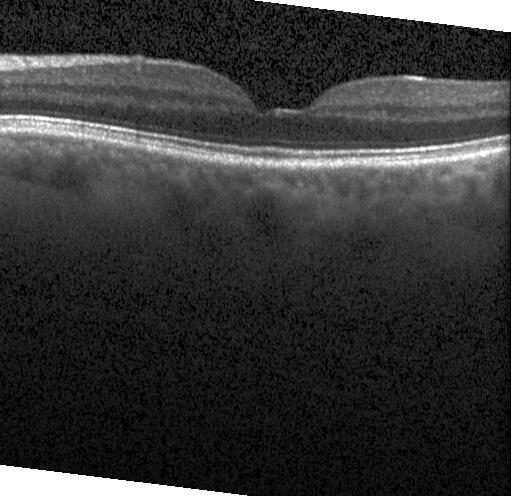 Optical coherence tomography B-scan — No evidence of choroidal neovascularization, diabetic macular edema, or drusen.